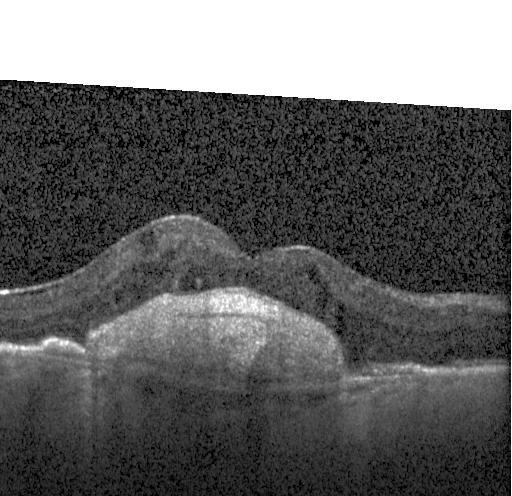
Spectral-domain optical coherence tomography · OCT line scan.
Diagnosis: a choroidal neovascular membrane.